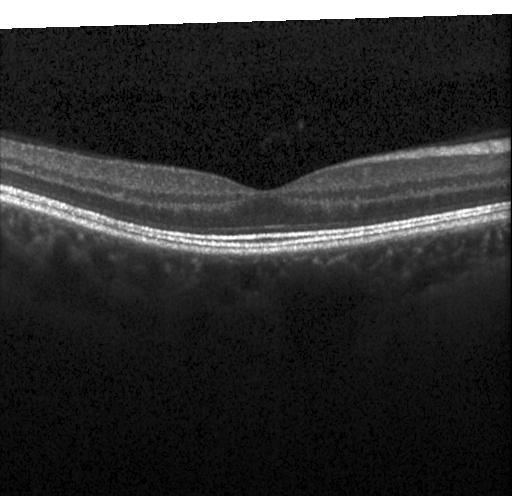 OCT B-scan
Finding: no CNV, DME, or drusen.